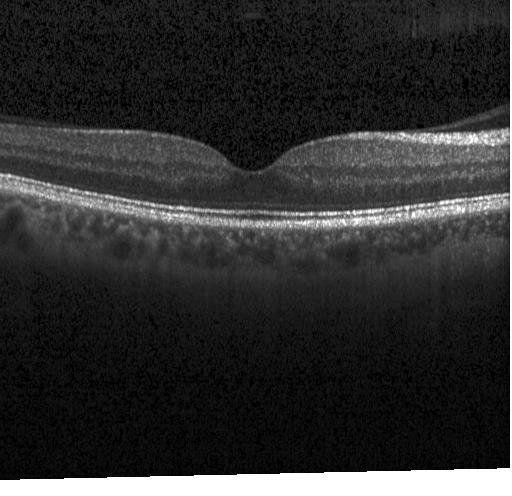 OCT B-scan — Diagnosis: no evidence of choroidal neovascularization, diabetic macular edema, or drusen.